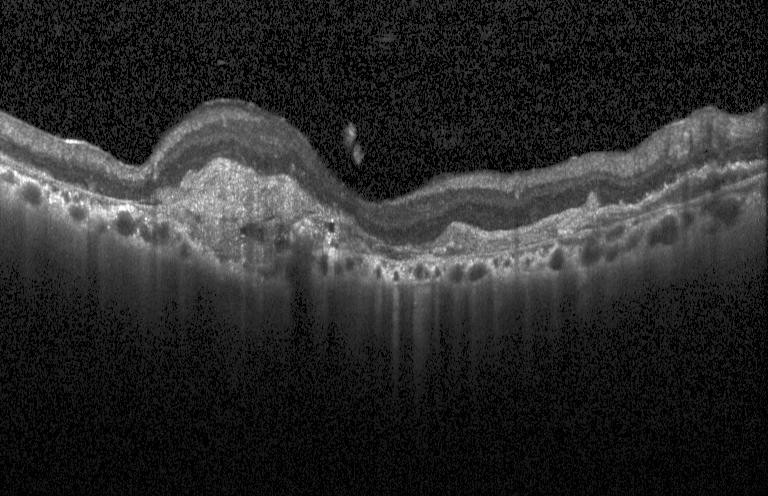

Macular scan, Heidelberg Spectralis, OCT B-scan — A choroidal neovascular membrane.